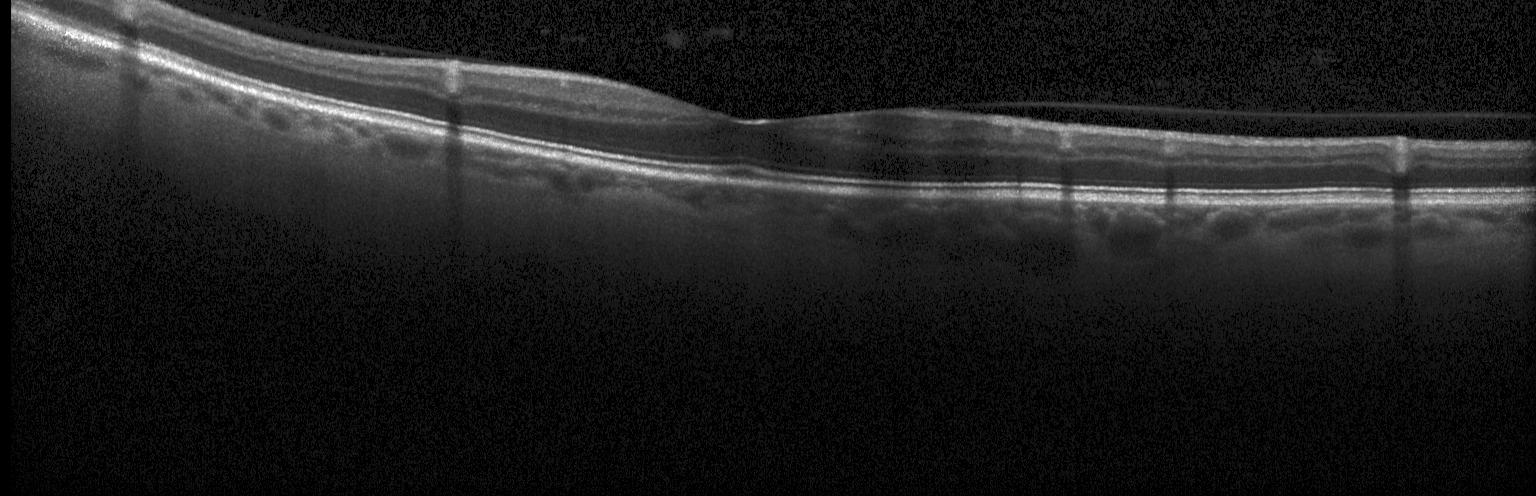 Impression: neither choroidal neovascularization, diabetic macular edema, nor drusen.